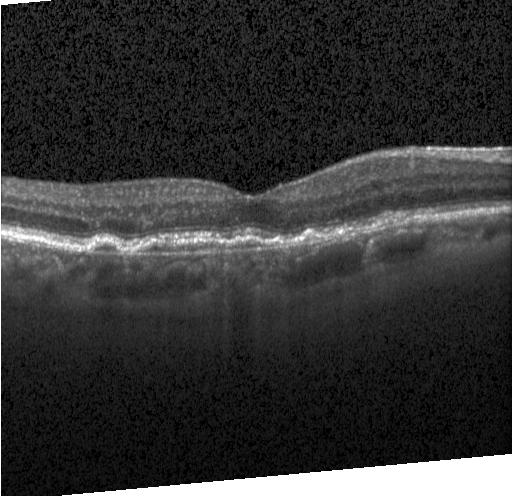
Heidelberg Spectralis OCT system; spectral-domain OCT; OCT B-scan
Impression: choroidal neovascularization (CNV).